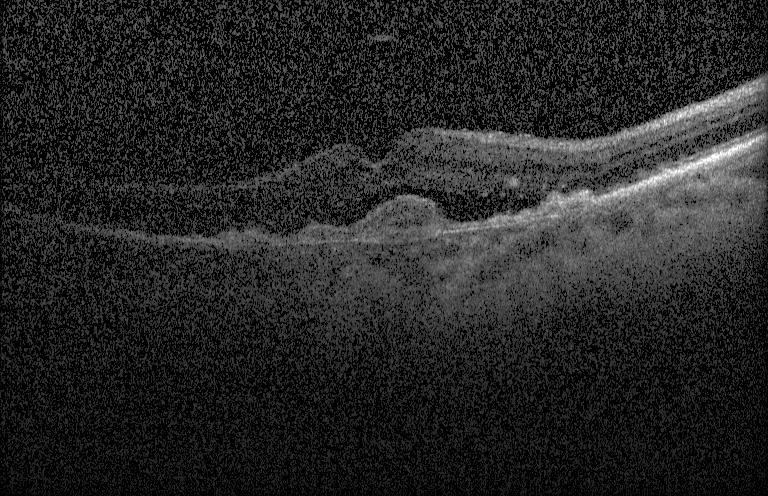

Spectral-domain OCT B-scan: choroidal neovascularization.